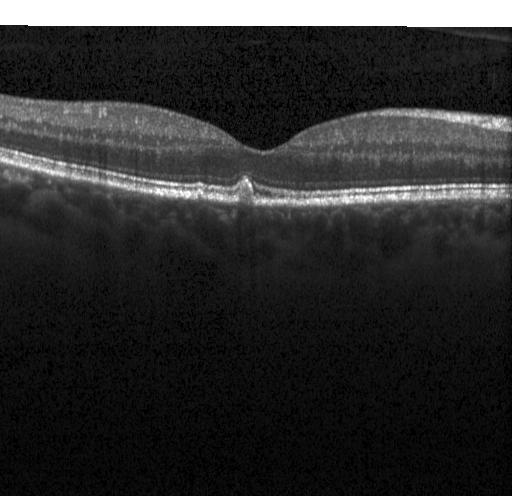

Retinal OCT B-scan, SD-OCT, Heidelberg Spectralis OCT system — Impression: multiple drusen.